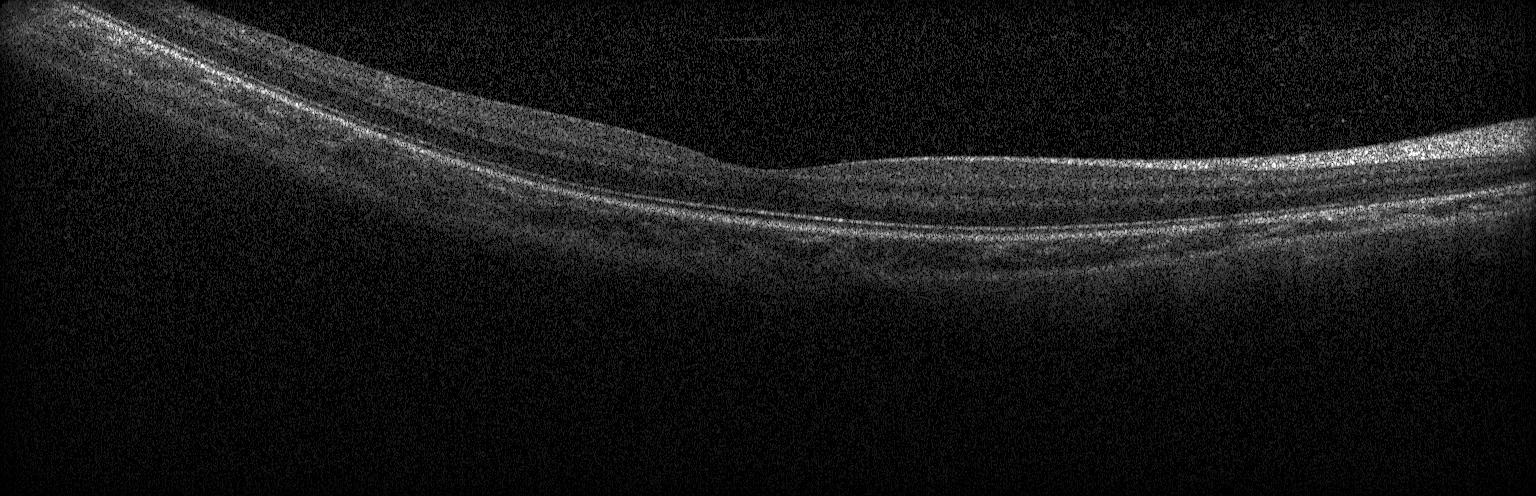 Macular OCT demonstrating no evidence of CNV, DME, or drusen.